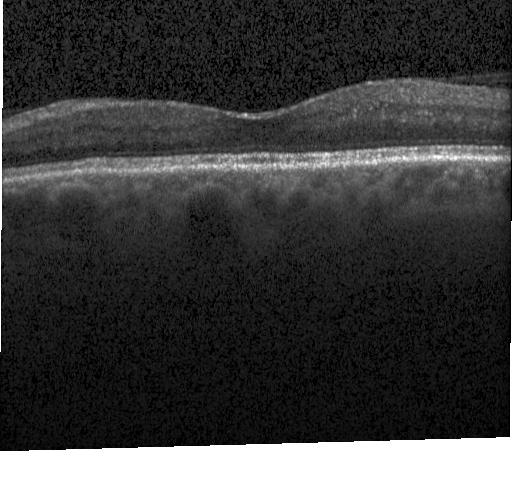

Through the macula, retinal OCT B-scan, instrument: Heidelberg Spectralis — Macular OCT: neither choroidal neovascularization, diabetic macular edema, nor drusen.